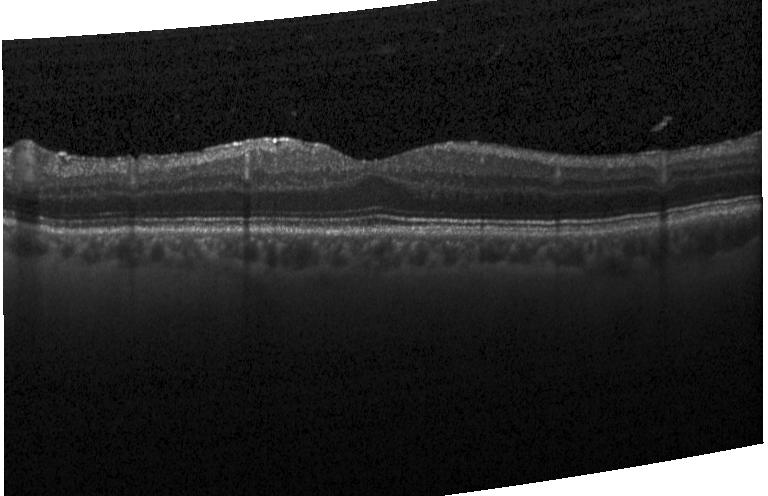 Diagnosis: no choroidal neovascularization, no diabetic macular edema, and no drusen.